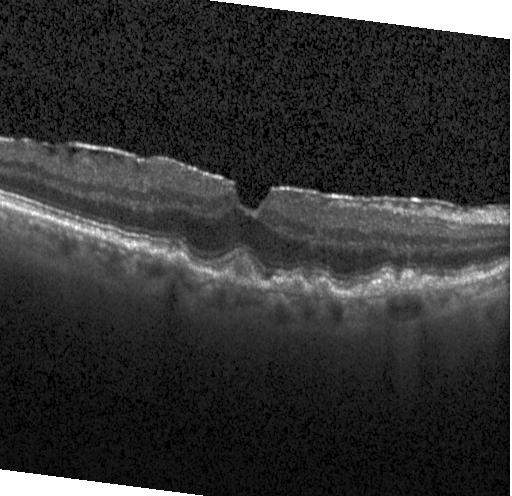 Retinal OCT B-scan. Dx: multiple drusen.